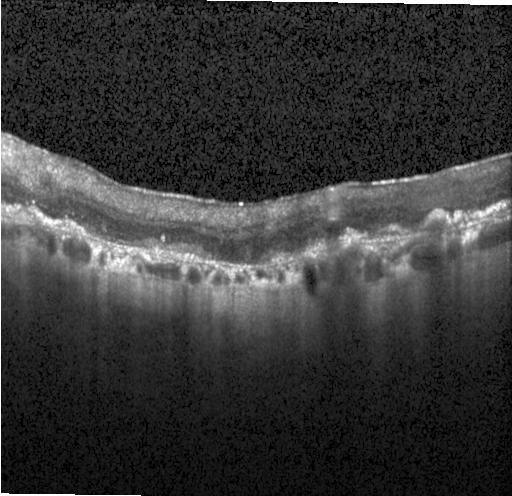

OCT B-scan, through the macula, SD-OCT, acquired on a Heidelberg Spectralis
The scan shows a choroidal neovascular membrane.